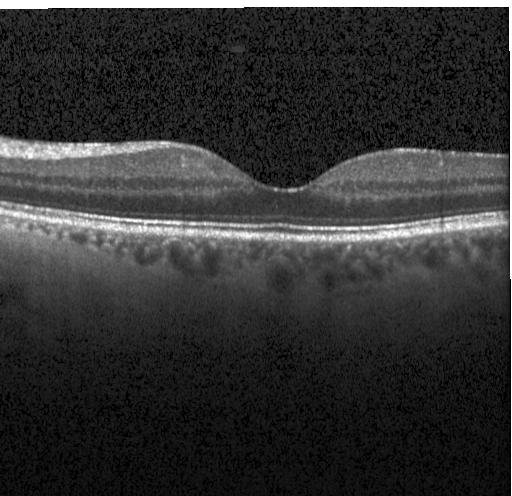

Optical coherence tomography B-scan
No choroidal neovascularization, diabetic macular edema, or drusen.